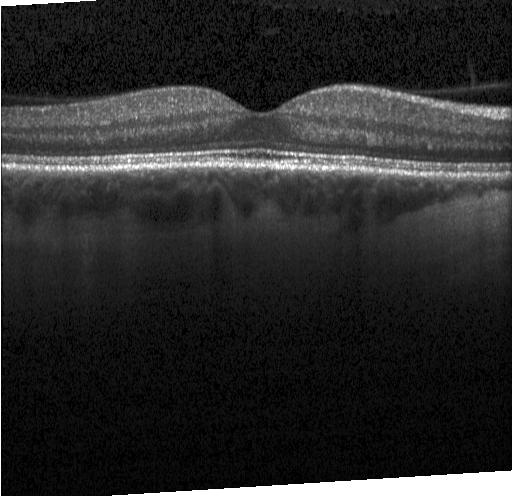
Diagnosis: no CNV, DME, or drusen.